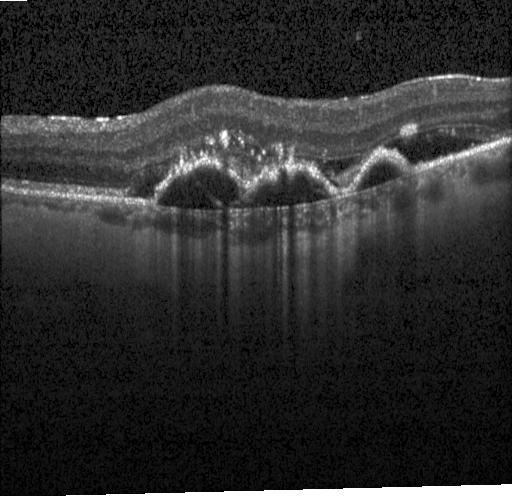 The scan shows choroidal neovascularization (CNV).